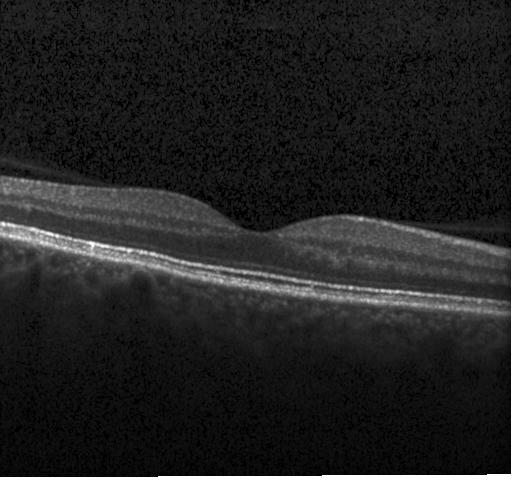

OCT line scan.
Impression: neither CNV, DME, nor drusen.